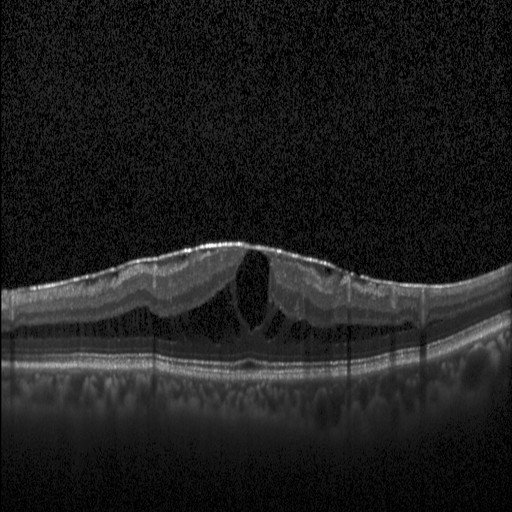

Retinal OCT cross-section — Finding: diabetic macular edema (DME).